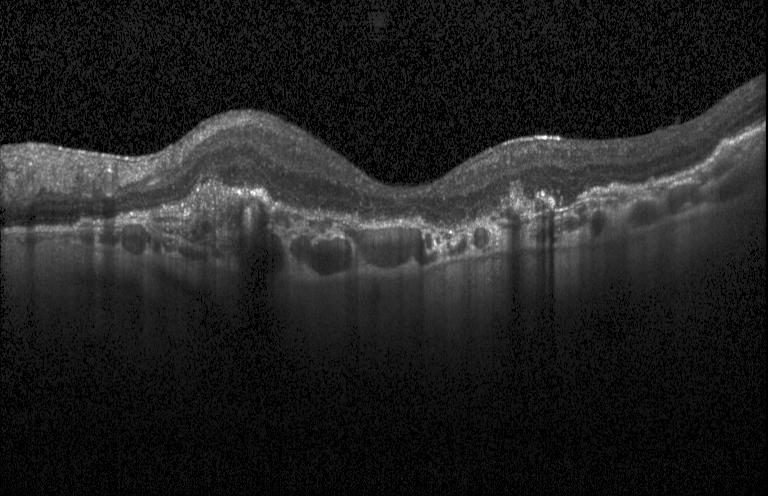

Instrument: Heidelberg Spectralis · retinal OCT cross-section. OCT finding: a choroidal neovascular membrane.